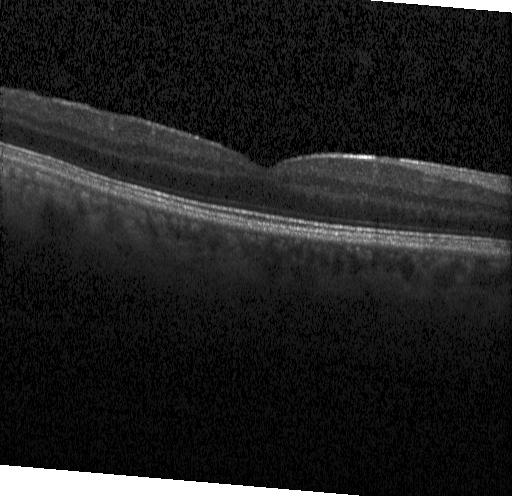

OCT line scan
Impression: no choroidal neovascularization, no diabetic macular edema, and no drusen.